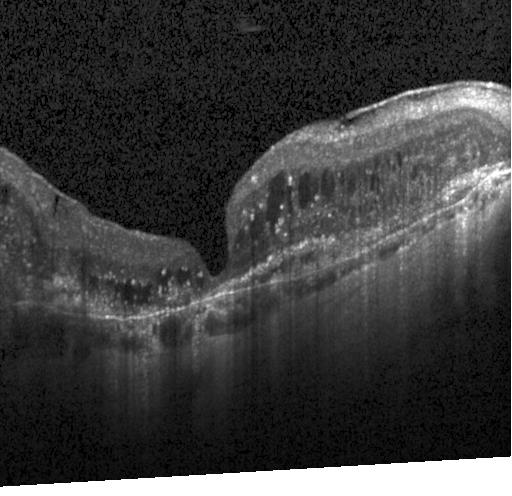
Optical coherence tomography B-scan. Assessment: a choroidal neovascular membrane.